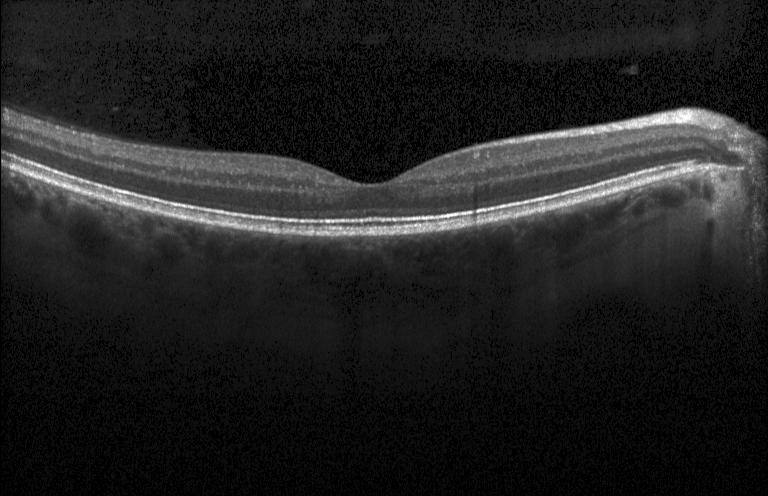

Spectral-domain OCT. Centered on the fovea. Heidelberg Spectralis. OCT B-scan — Finding: no CNV, no DME, and no drusen.